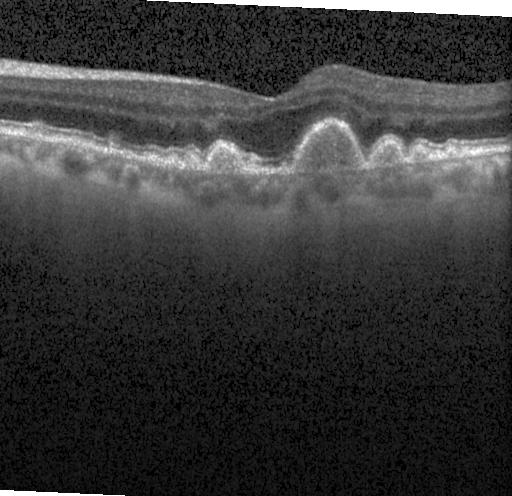

Retinal OCT B-scan. Drusen.